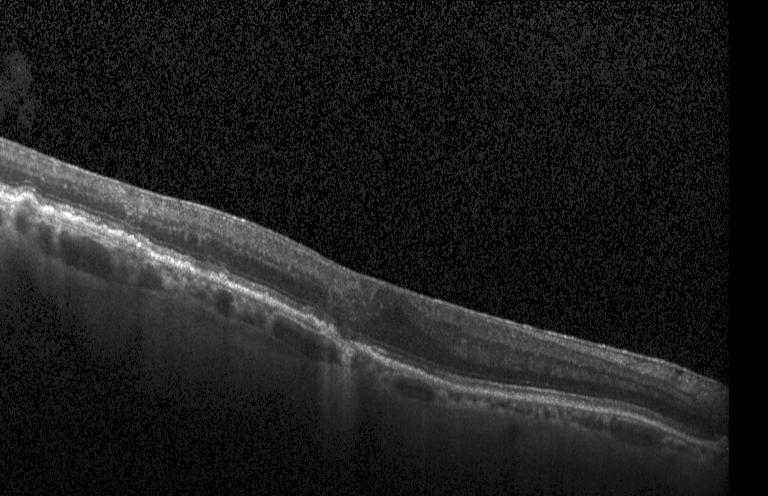 OCT line scan · Heidelberg Spectralis · SD-OCT.
Diagnosis: a choroidal neovascular membrane.